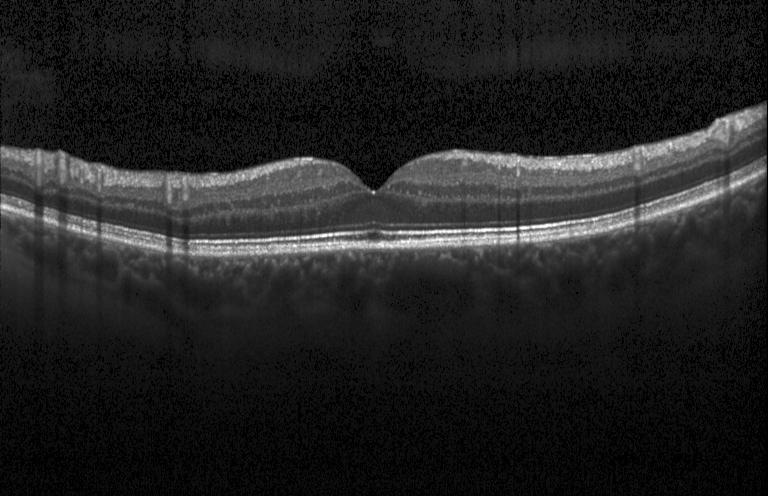

Retinal OCT cross-section
This B-scan demonstrates neither choroidal neovascularization, diabetic macular edema, nor drusen.